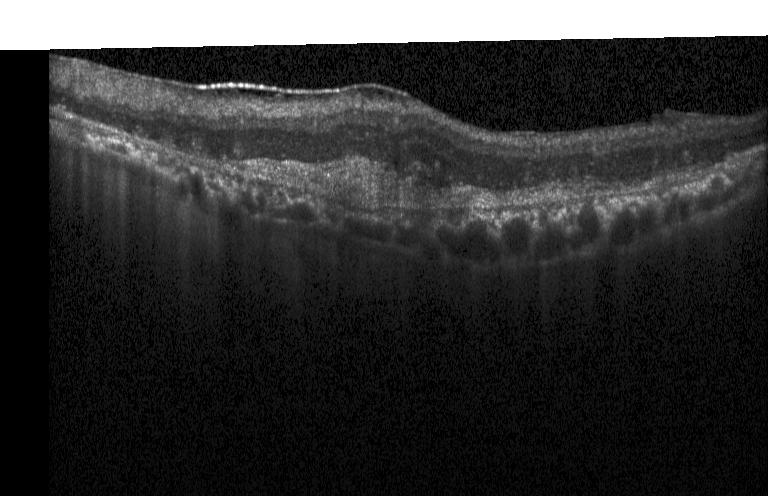 Retinal OCT B-scan; macular scan
Finding: CNV.